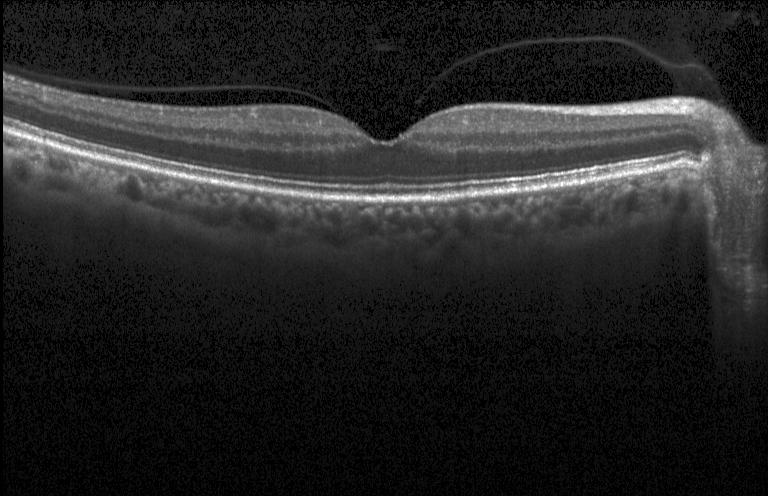 Impression: no CNV, DME, or drusen.